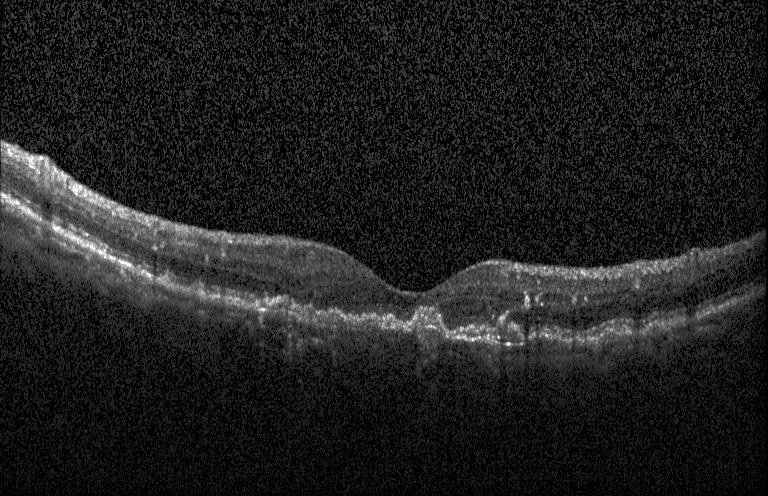 Dx: a choroidal neovascular membrane.